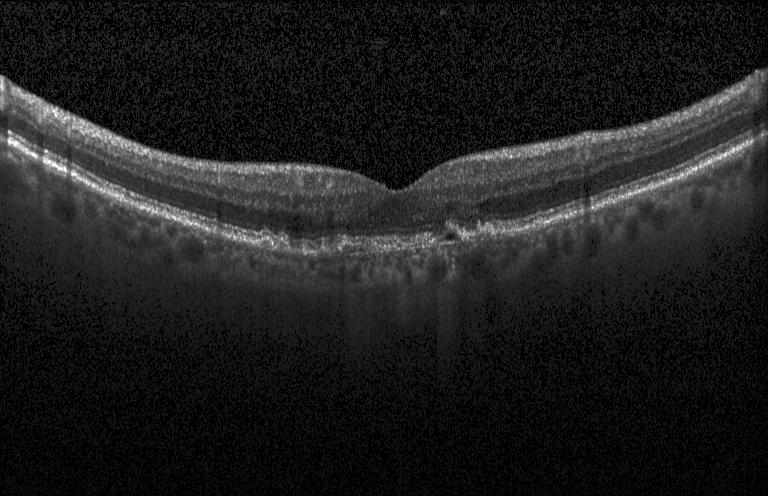
Centered on the fovea · Heidelberg Spectralis · SD-OCT · optical coherence tomography scan — The scan shows a choroidal neovascular membrane.